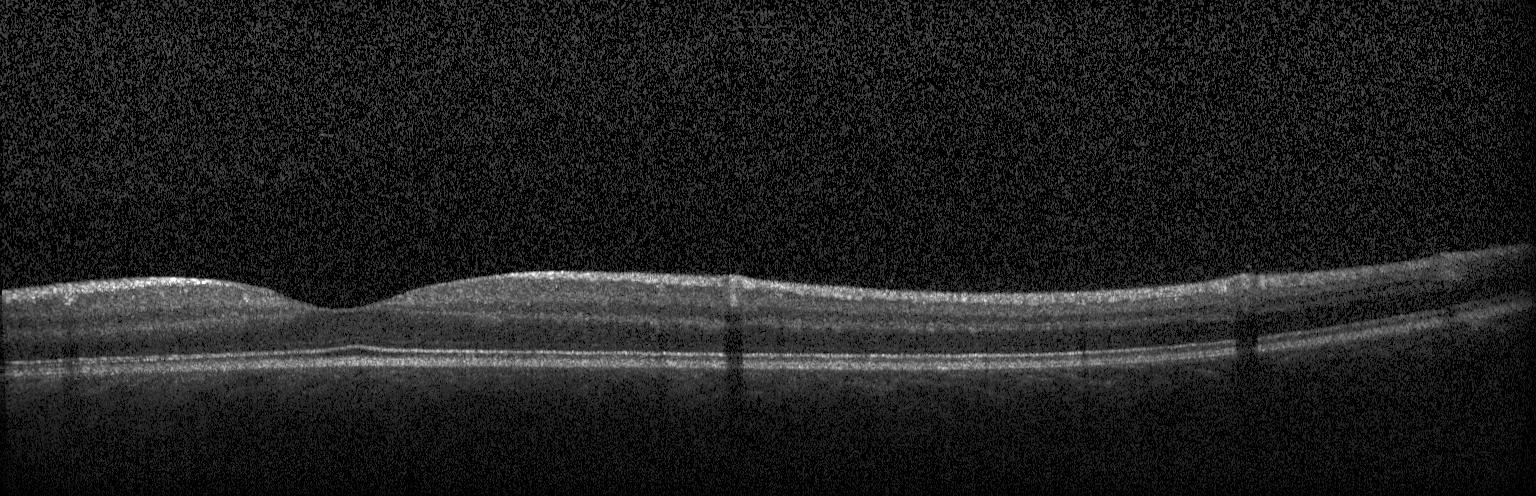 Through the macula, spectral-domain optical coherence tomography, OCT B-scan, Heidelberg Spectralis OCT system — Finding: no evidence of CNV, DME, or drusen.